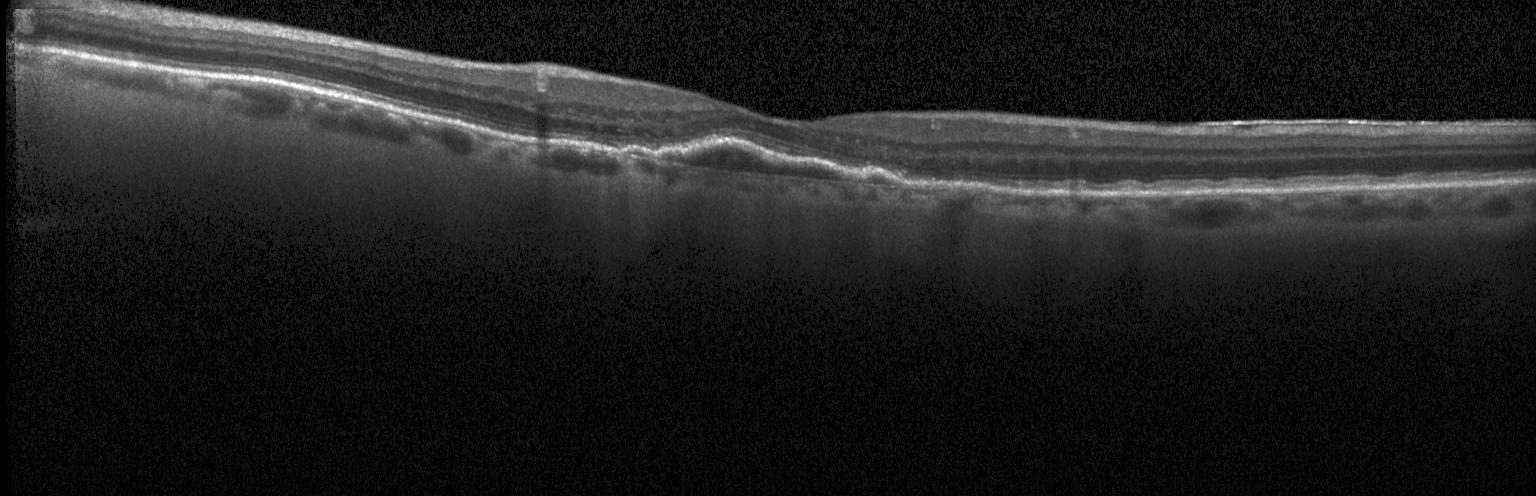
Diagnosis: CNV.